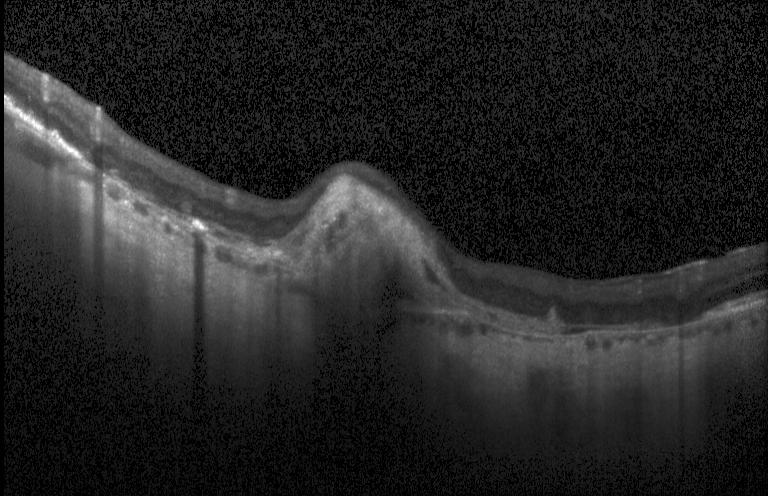

OCT finding: a choroidal neovascular membrane.